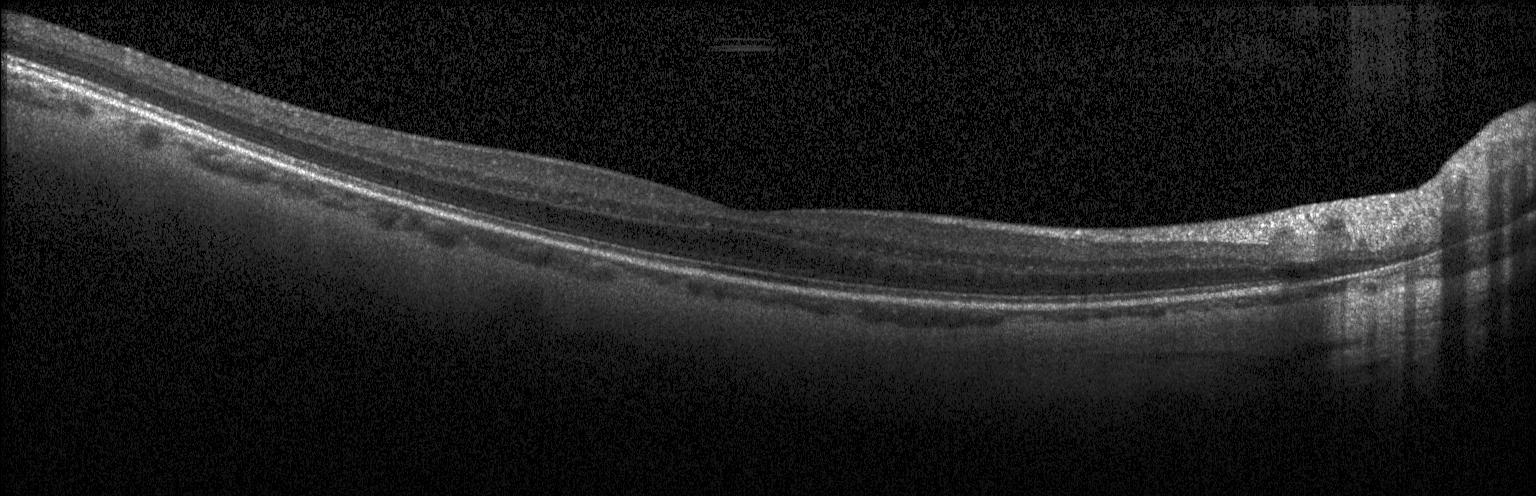

Diagnosis: neither choroidal neovascularization, diabetic macular edema, nor drusen.